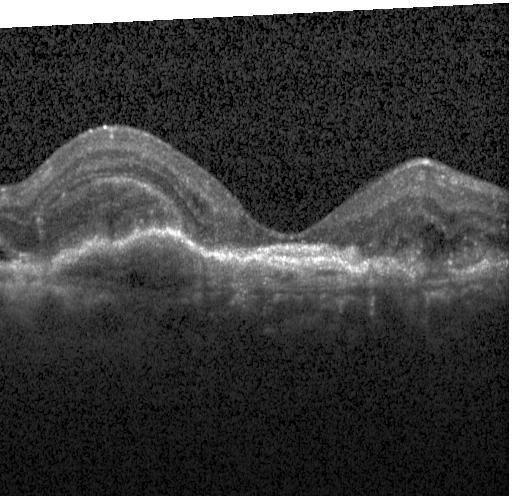 Diagnosis: a choroidal neovascular membrane.